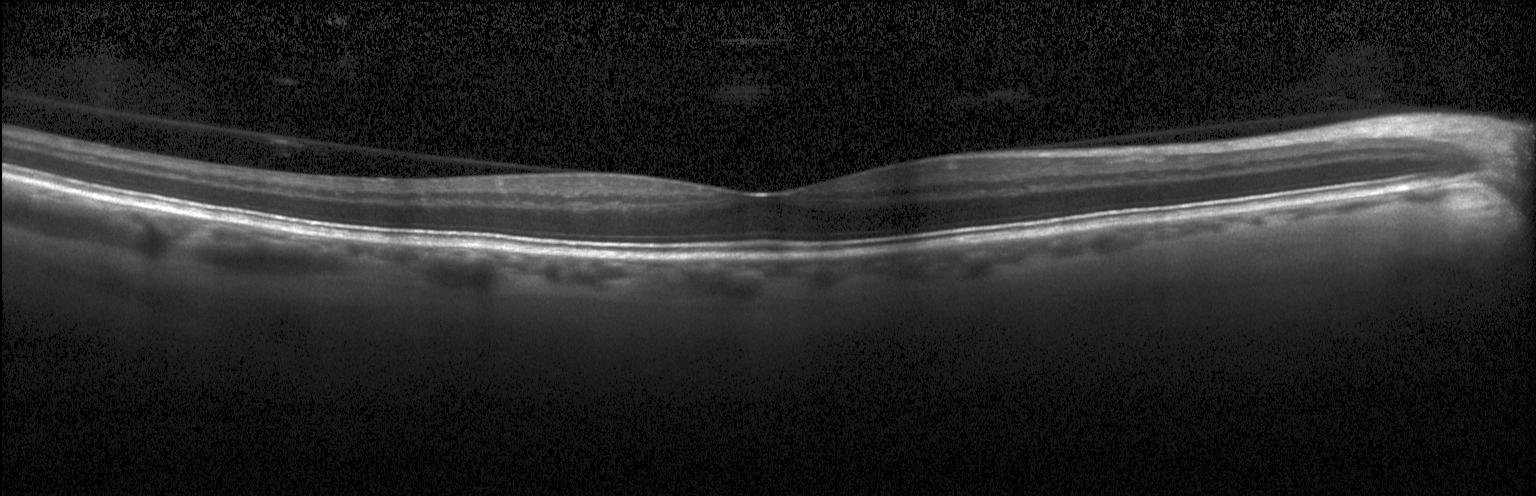
Finding: neither CNV, DME, nor drusen.